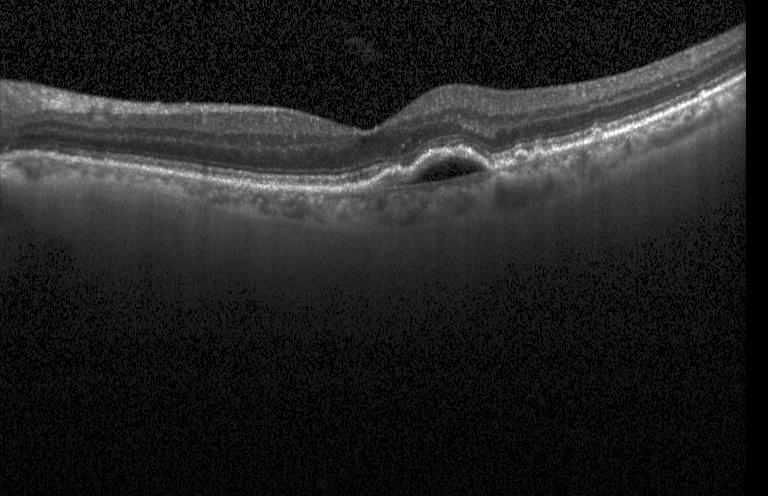 SD-OCT; horizontal scan through the fovea; OCT B-scan; Heidelberg Spectralis
Assessment: a choroidal neovascular membrane.